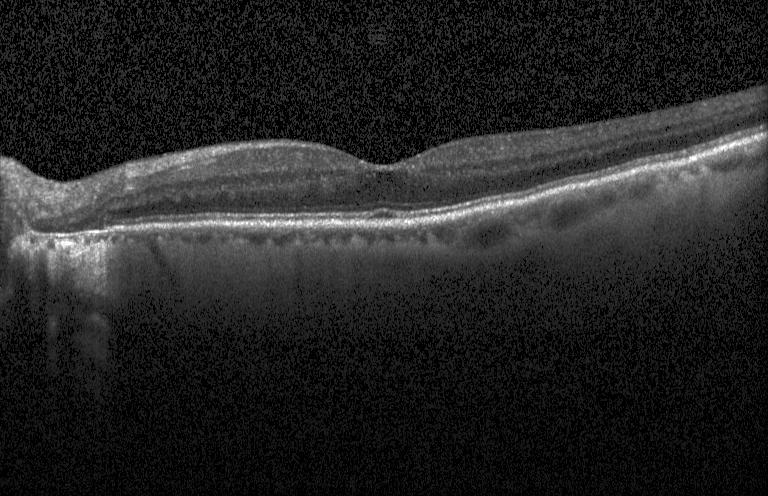

Retinal OCT cross-section — OCT finding: no CNV, DME, or drusen.